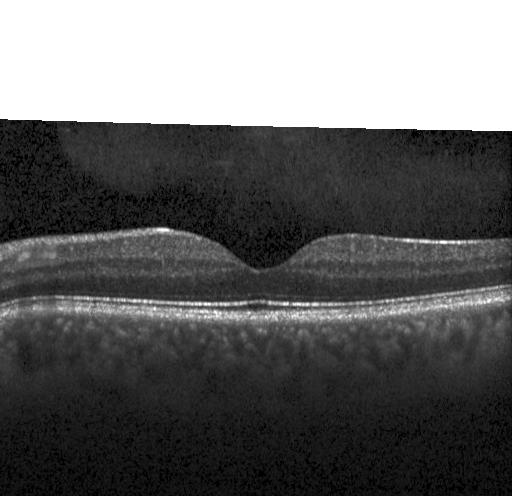

Macular OCT: no evidence of CNV, DME, or drusen.